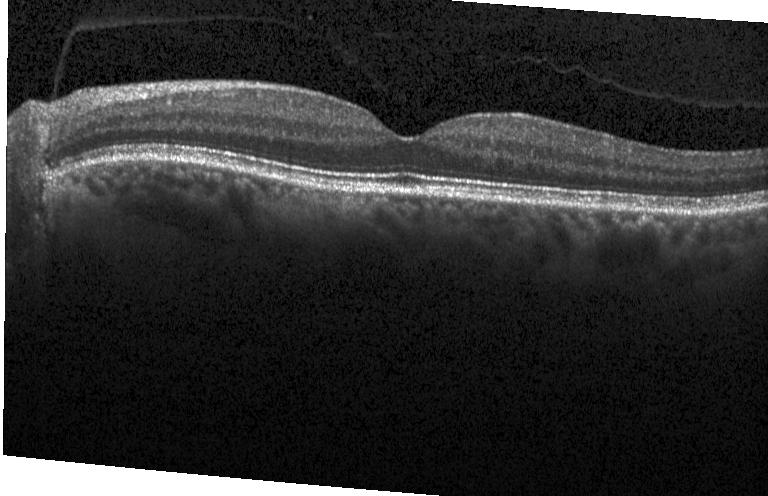
Optical coherence tomography B-scan.
Macular OCT: no choroidal neovascularization, no diabetic macular edema, and no drusen.